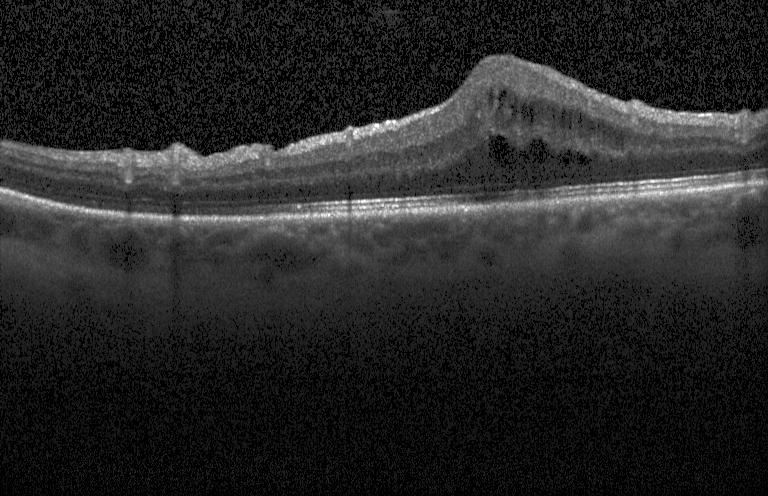
Retinal OCT B-scan. Finding: DME.